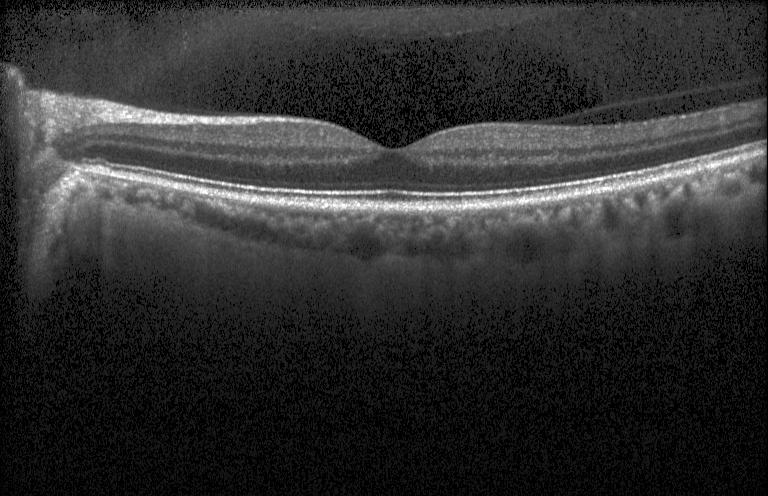
Retinal OCT cross-section, Heidelberg Spectralis. Macular OCT: no choroidal neovascularization, no diabetic macular edema, and no drusen.